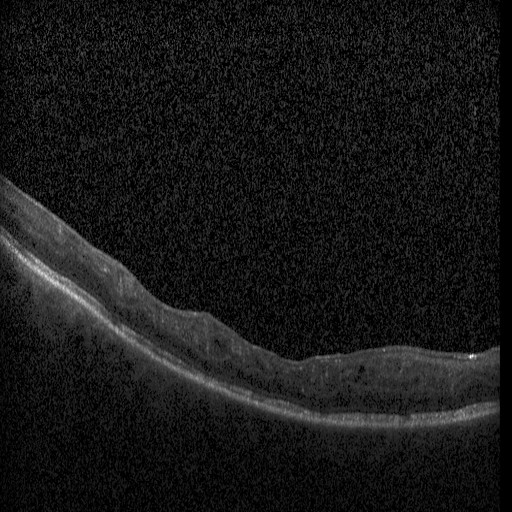
Optical coherence tomography scan · fovea-centered
Diagnosis: diabetic macular edema (DME).